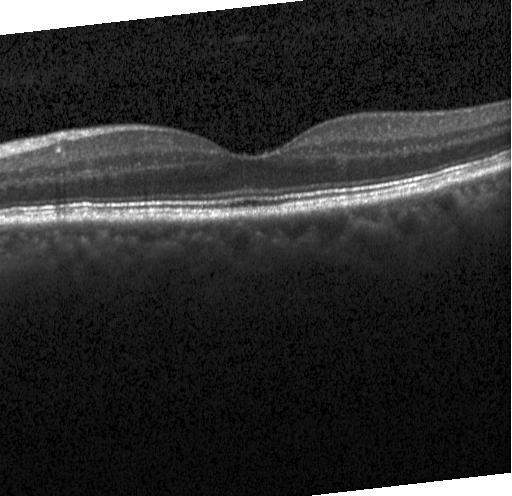

Heidelberg Spectralis OCT system · OCT B-scan
The scan shows no evidence of choroidal neovascularization, diabetic macular edema, or drusen.